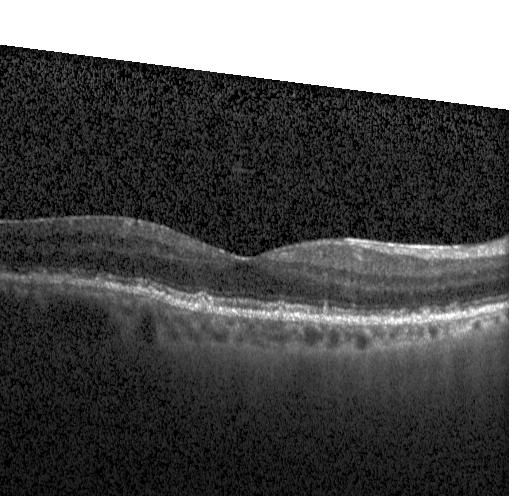 Retinal OCT cross-section. Acquired on a Heidelberg Spectralis — Assessment: drusen.